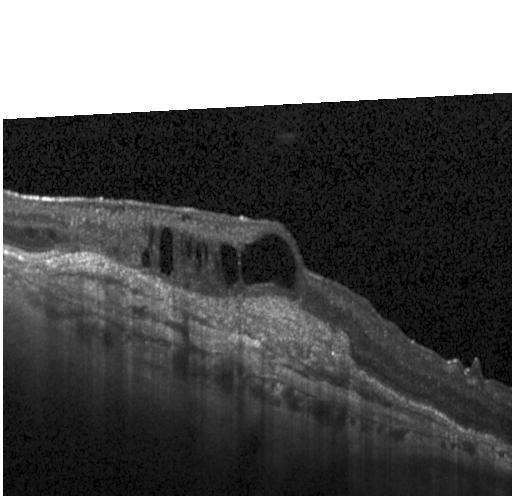

Spectral-domain optical coherence tomography, OCT B-scan, instrument: Heidelberg Spectralis, fovea-centered
Diagnosis: a choroidal neovascular membrane.